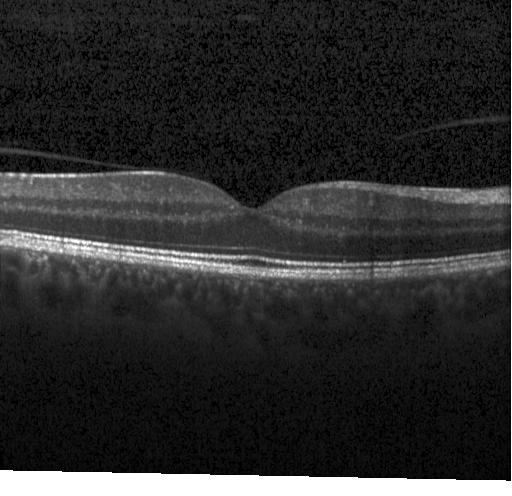

Retinal OCT cross-section · Heidelberg Spectralis · SD-OCT — Assessment: no CNV, no DME, and no drusen.